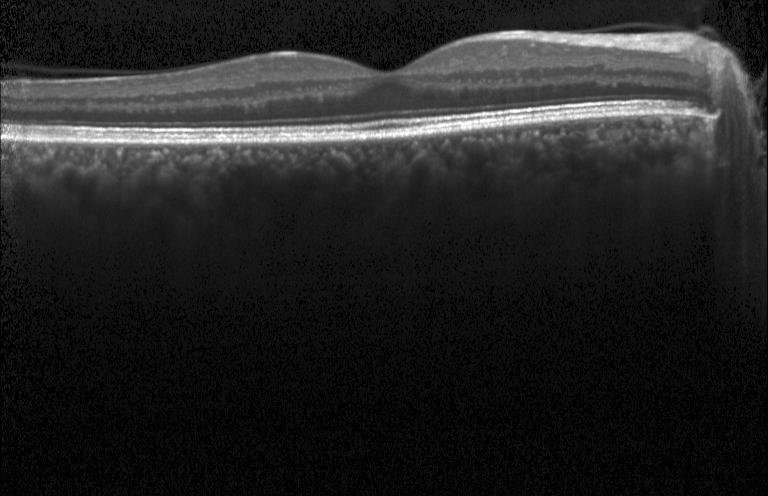
Diagnosis: no evidence of CNV, DME, or drusen.